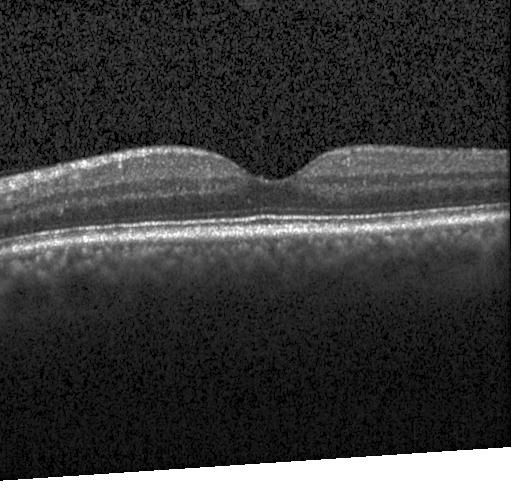

OCT B-scan showing neither CNV, DME, nor drusen.